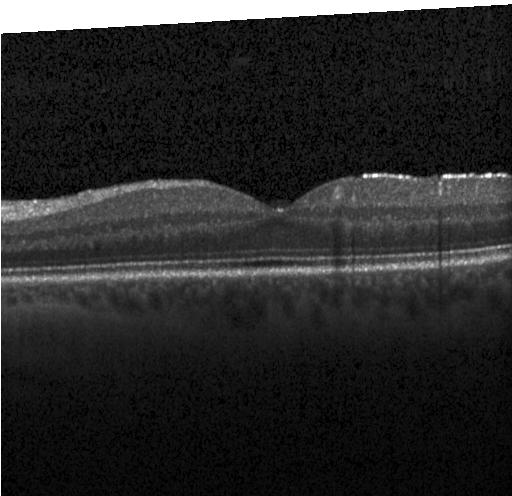

Horizontal scan through the fovea. Optical coherence tomography B-scan. Heidelberg Spectralis — This B-scan demonstrates no evidence of CNV, DME, or drusen.